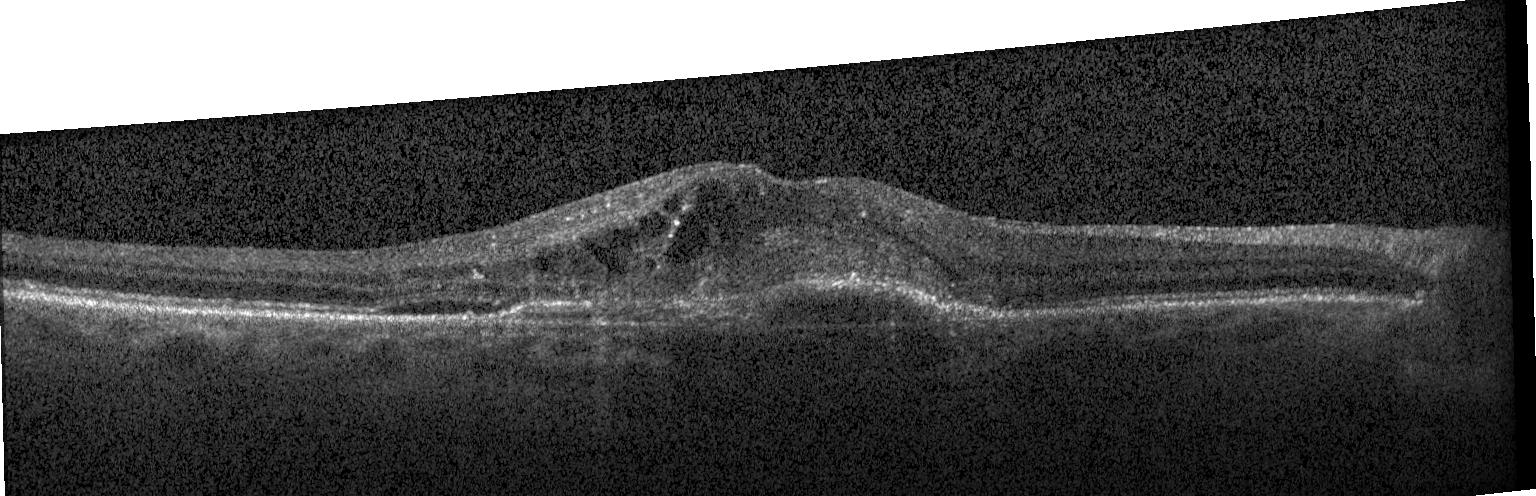

Through the macula; optical coherence tomography B-scan; spectral-domain OCT
OCT finding: choroidal neovascularization.